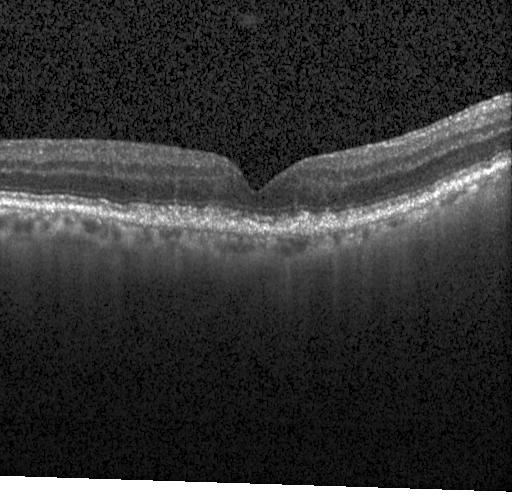 The scan shows drusen.